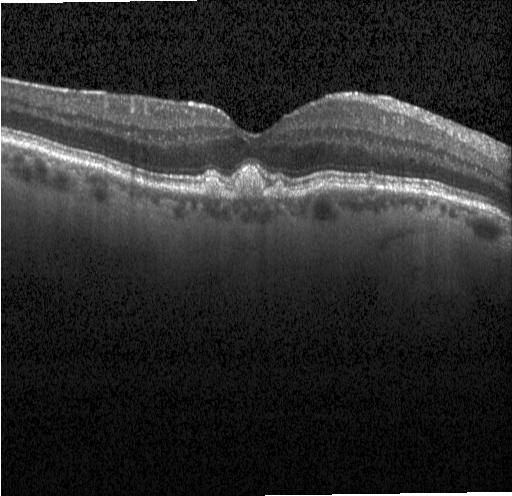 OCT finding: sub-RPE drusenoid deposits.